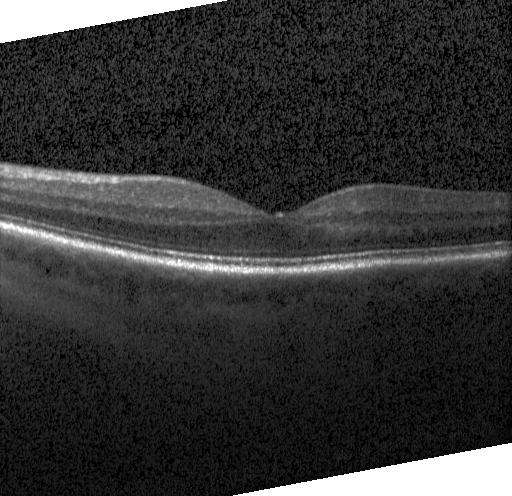 Retinal OCT cross-section · spectral-domain OCT · horizontal scan through the fovea.
Macular OCT: no CNV, DME, or drusen.